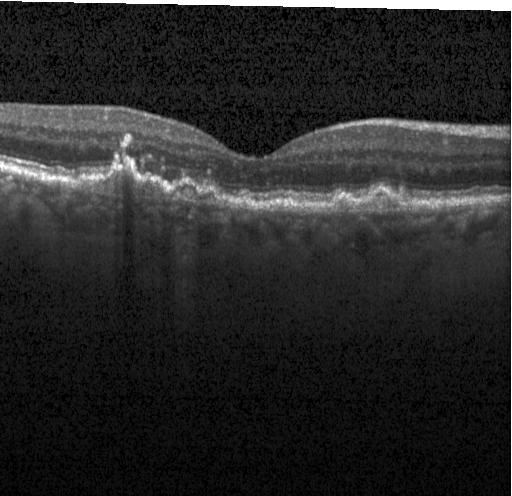
Macular OCT demonstrating a choroidal neovascular membrane.